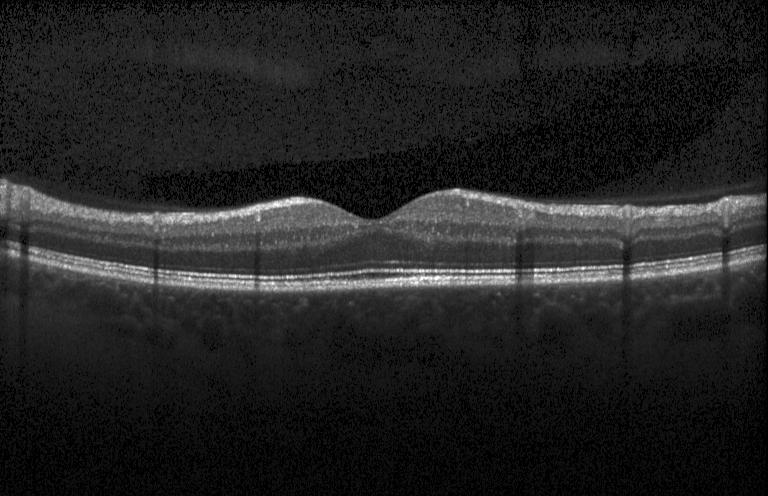
OCT line scan — OCT finding: no choroidal neovascularization, no diabetic macular edema, and no drusen.